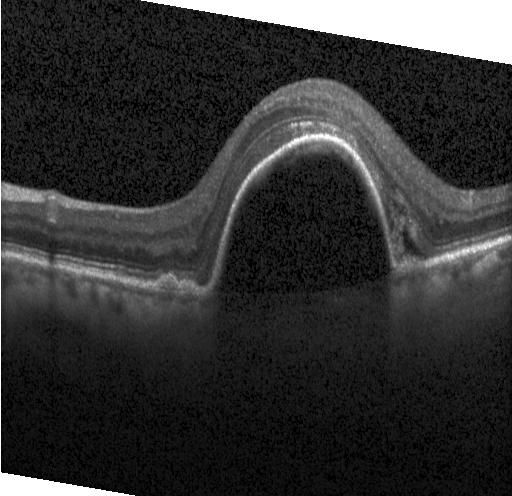
Impression: choroidal neovascularization.